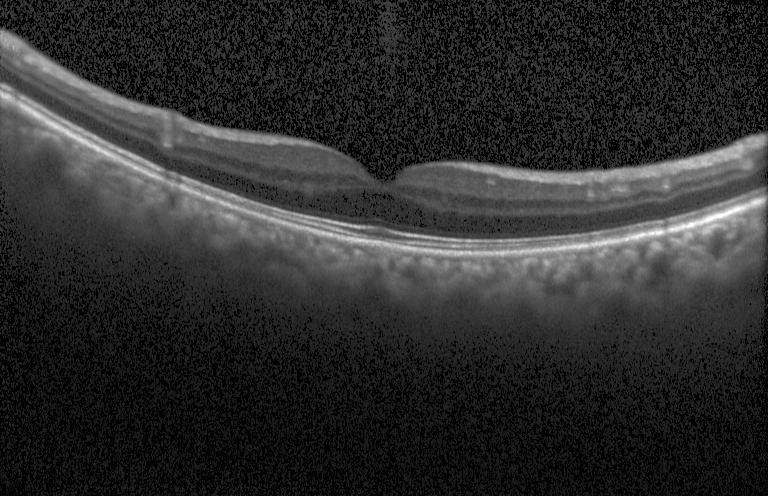

Diagnosis: no CNV, no DME, and no drusen.